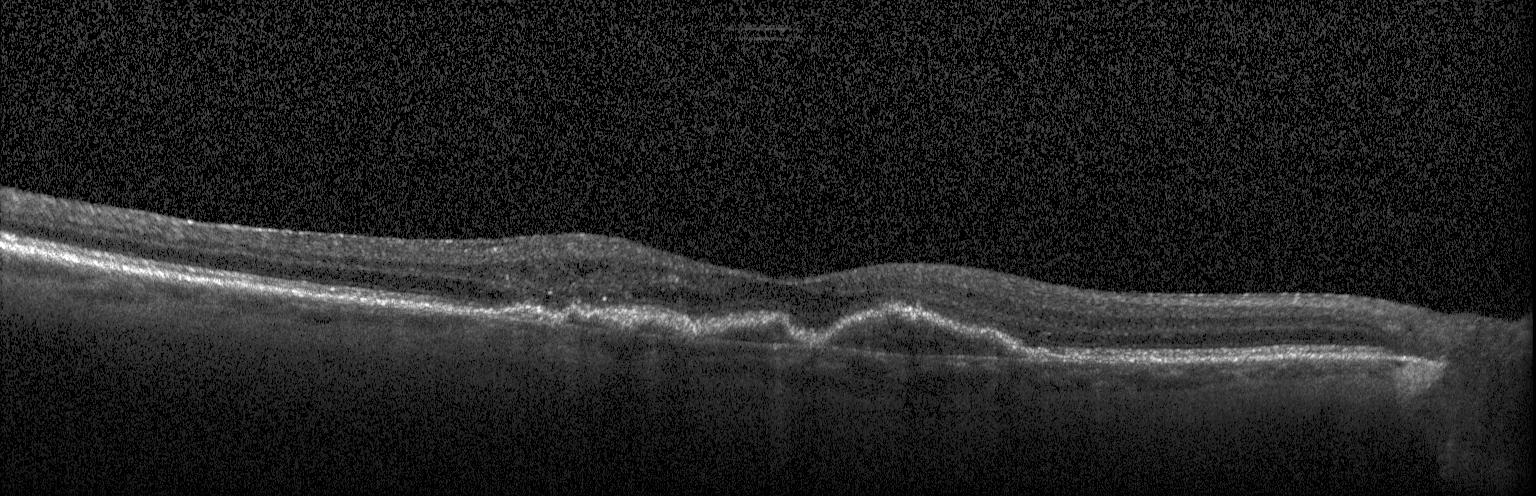
OCT B-scan showing a choroidal neovascular membrane.